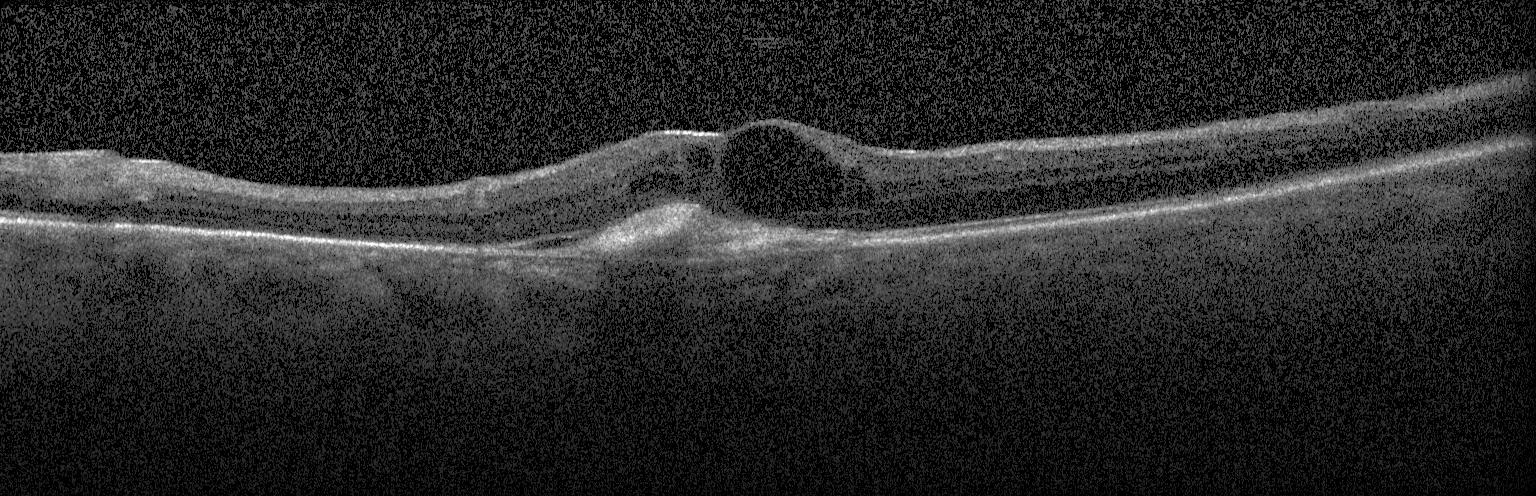 OCT line scan; horizontal scan through the fovea; Heidelberg Spectralis OCT system. OCT finding: a choroidal neovascular membrane.